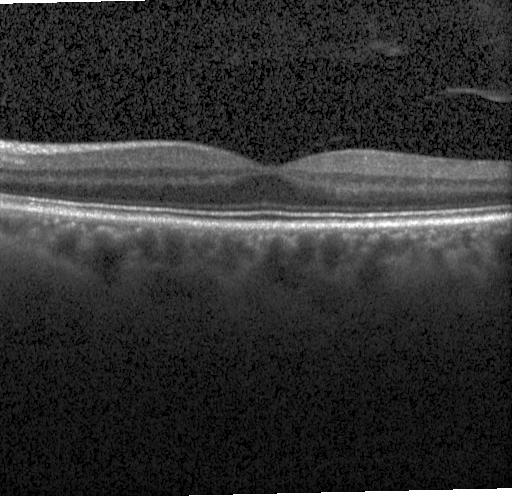 Finding: no CNV, no DME, and no drusen.